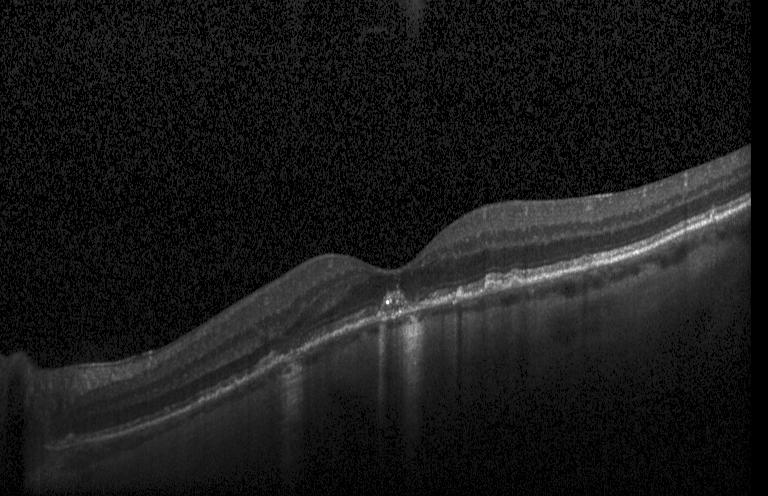

Instrument: Heidelberg Spectralis, optical coherence tomography B-scan, macular scan
Finding: choroidal neovascularization.